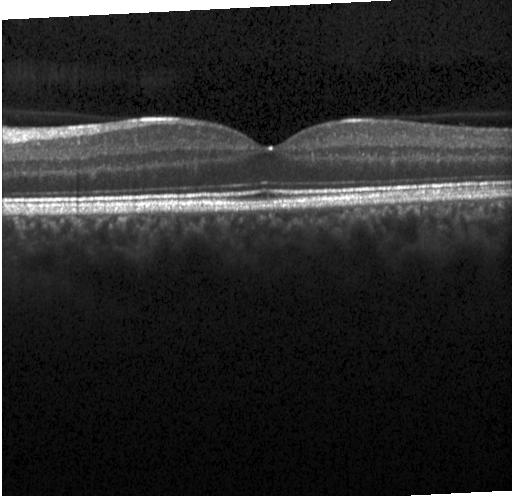

SD-OCT · Heidelberg Spectralis · through the macula · retinal OCT B-scan — The scan shows no choroidal neovascularization, no diabetic macular edema, and no drusen.